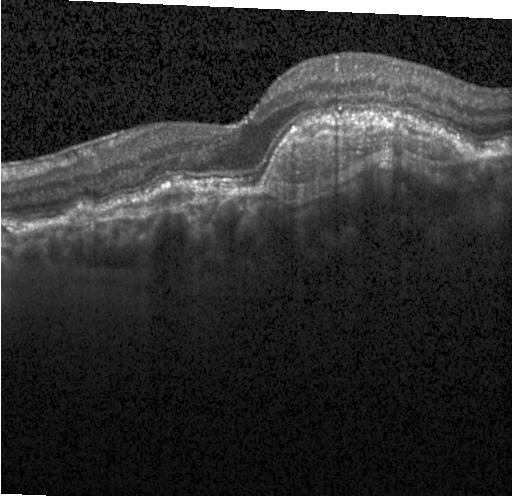 Centered on the fovea, optical coherence tomography B-scan, spectral-domain optical coherence tomography
Impression: a choroidal neovascular membrane.